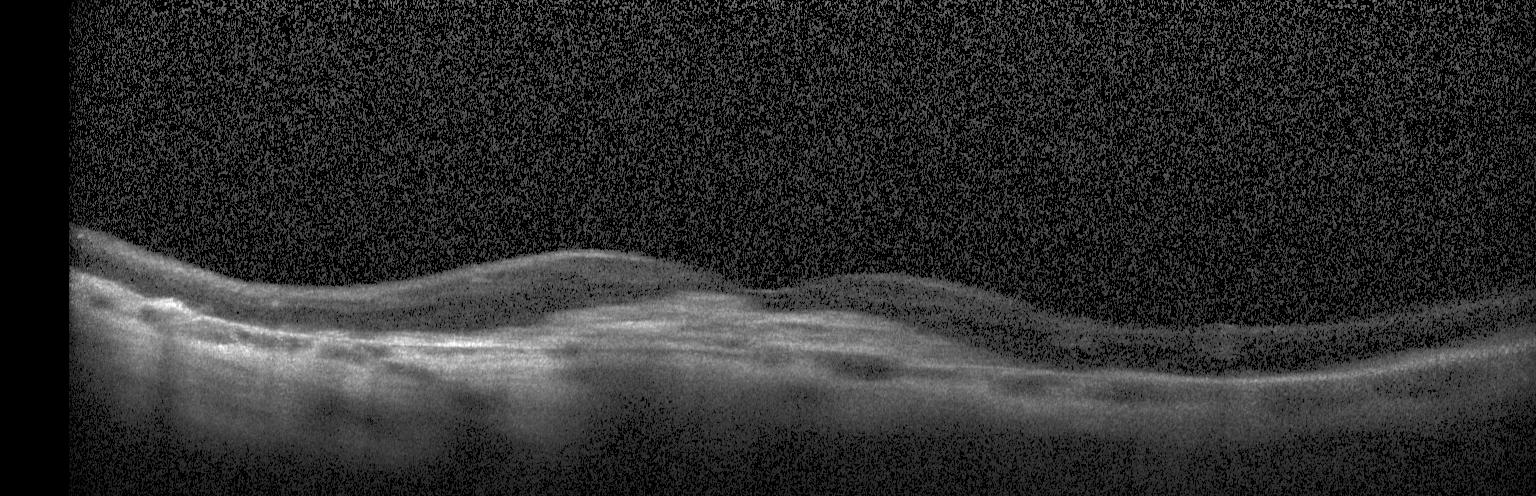

OCT scan showing choroidal neovascularization (CNV).